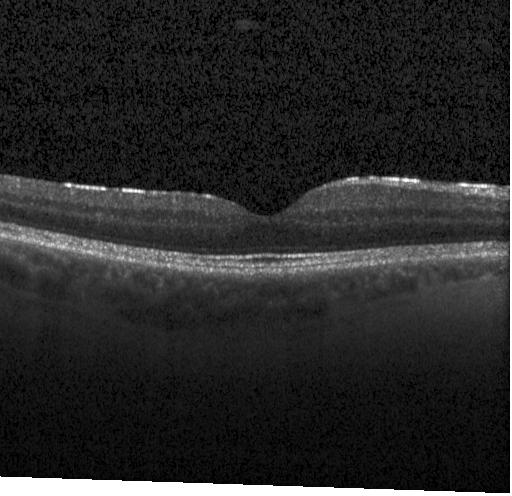 Finding: no CNV, DME, or drusen.